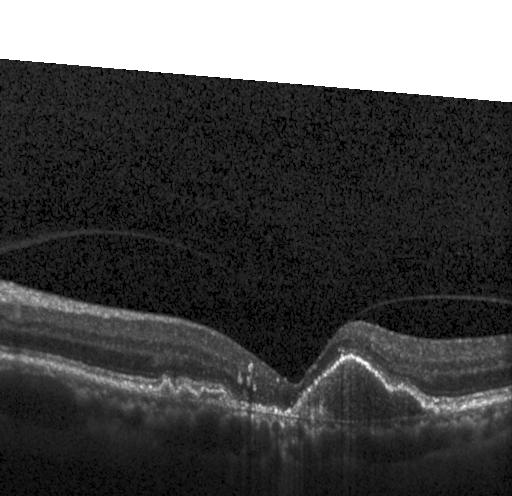 OCT finding: a choroidal neovascular membrane.